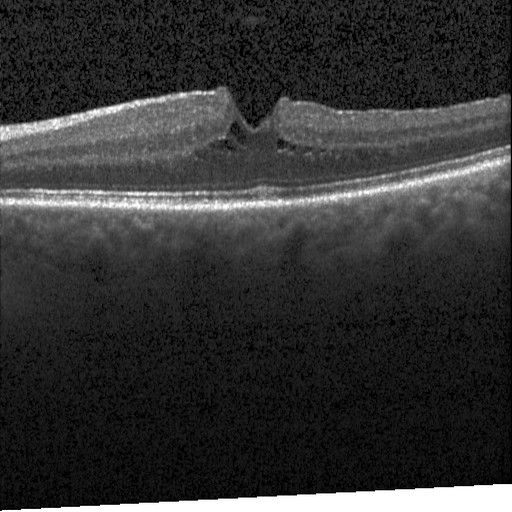 Spectral-domain OCT · Heidelberg Spectralis OCT system · optical coherence tomography scan · through the macula — Finding: diabetic macular edema.